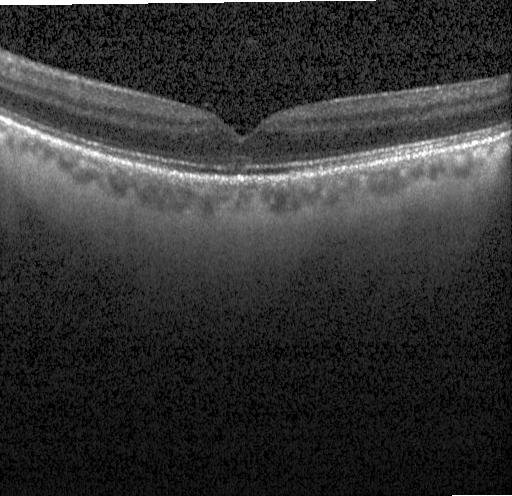
Retinal OCT cross-section; spectral-domain optical coherence tomography; acquired on a Heidelberg Spectralis. Diagnosis: no choroidal neovascularization, no diabetic macular edema, and no drusen.